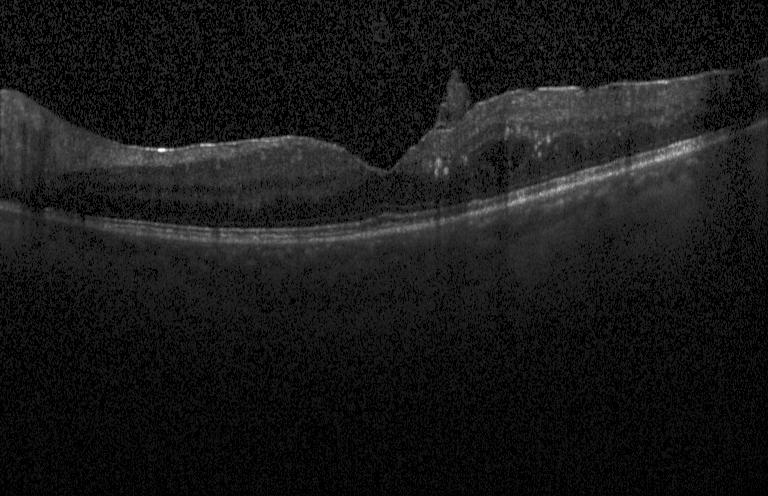

Dx: diabetic macular edema.